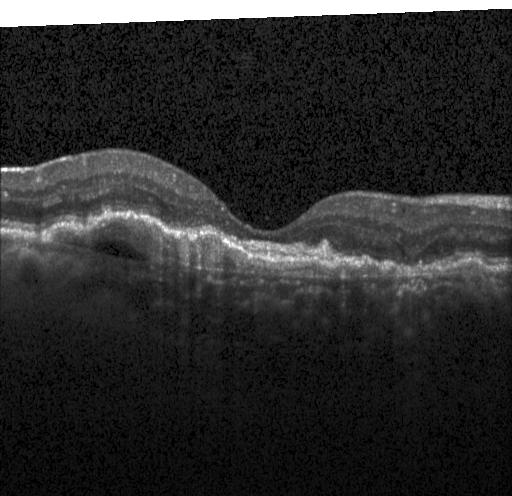 SD-OCT · retinal OCT cross-section · macular scan
OCT finding: a choroidal neovascular membrane.